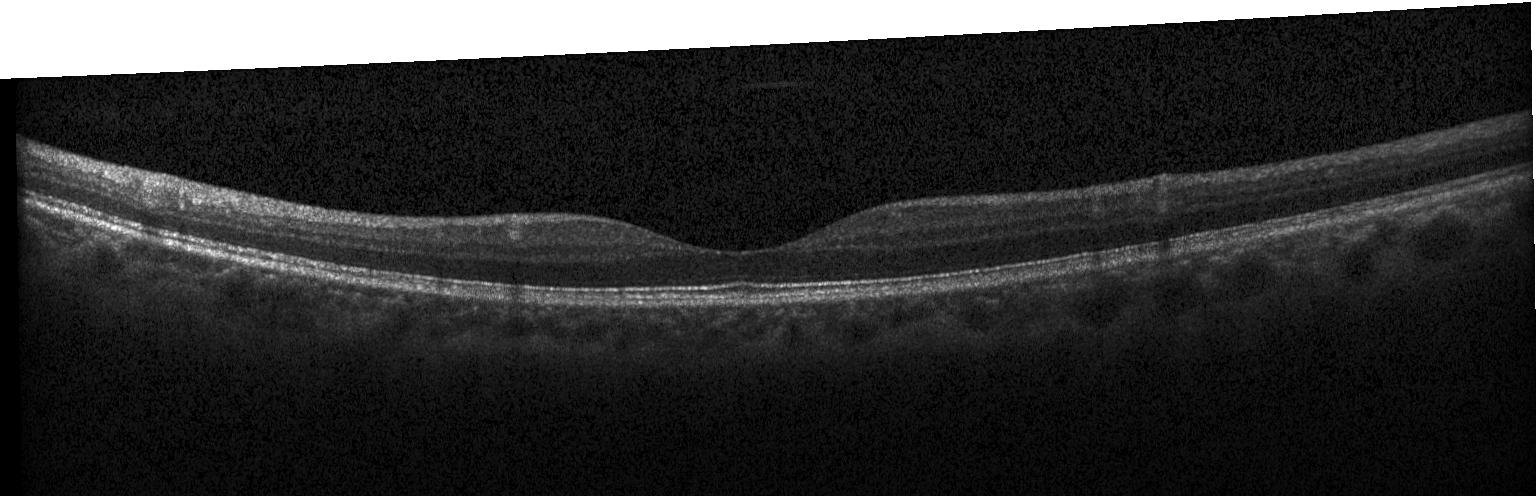 Impression: no CNV, no DME, and no drusen.